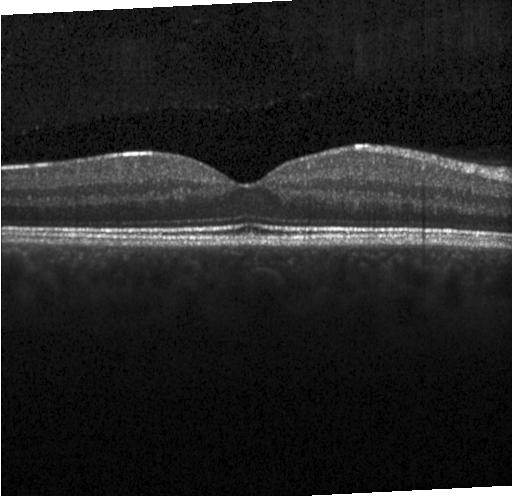
Through the macula · Heidelberg Spectralis · spectral-domain optical coherence tomography · OCT line scan — Finding: no choroidal neovascularization, no diabetic macular edema, and no drusen.